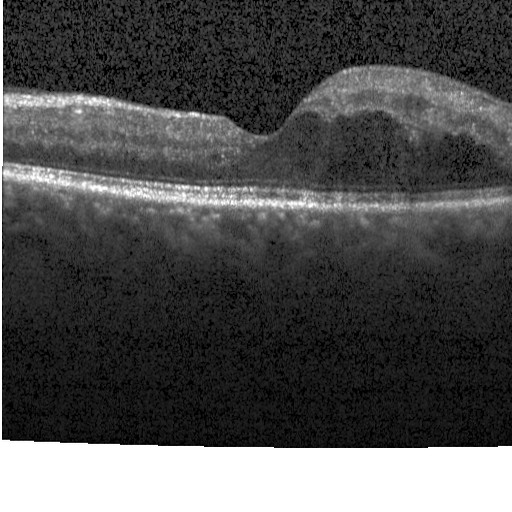
Retinal OCT B-scan — Finding: diabetic macular edema (DME).